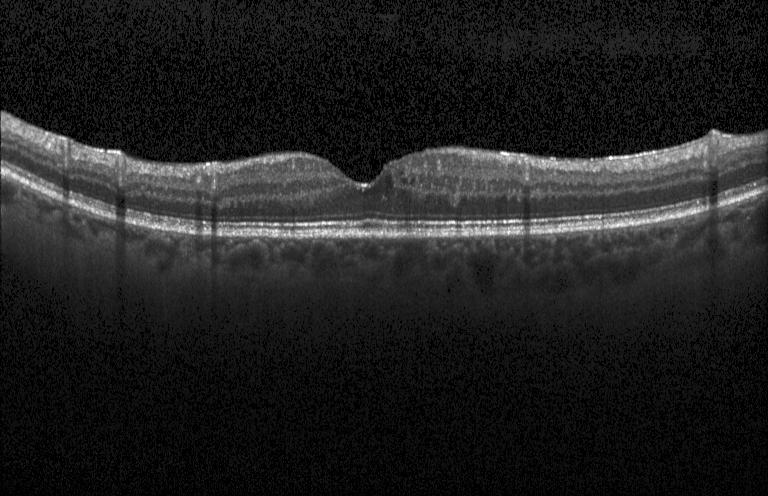
Finding: diabetic macular edema.